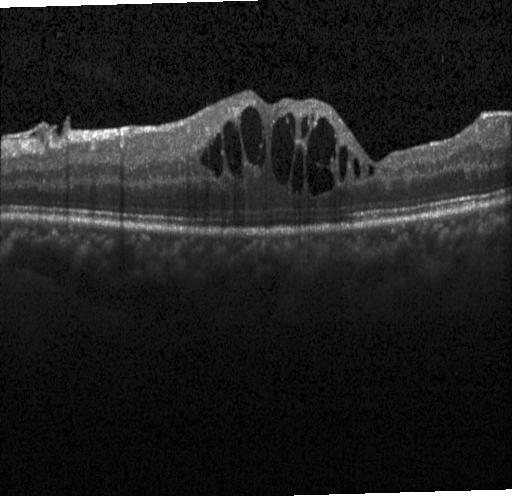 Heidelberg Spectralis OCT system · OCT line scan — Impression: diabetic macular edema.